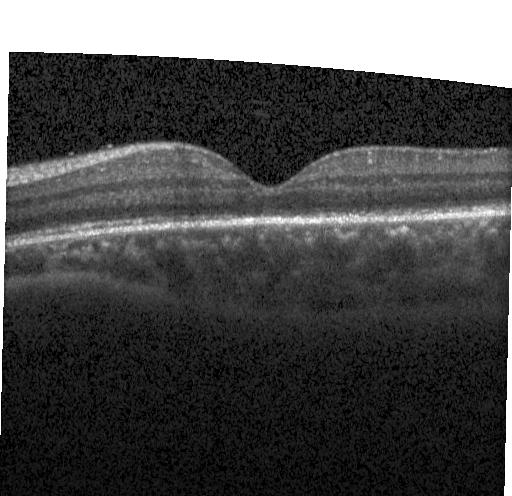
Finding: no CNV, DME, or drusen.